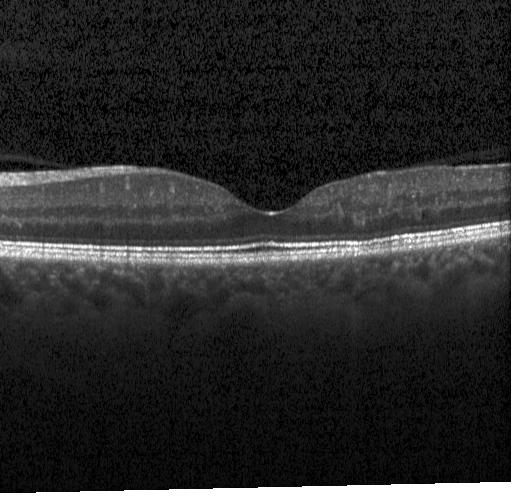

Spectral-domain OCT; retinal OCT cross-section
Assessment: neither choroidal neovascularization, diabetic macular edema, nor drusen.